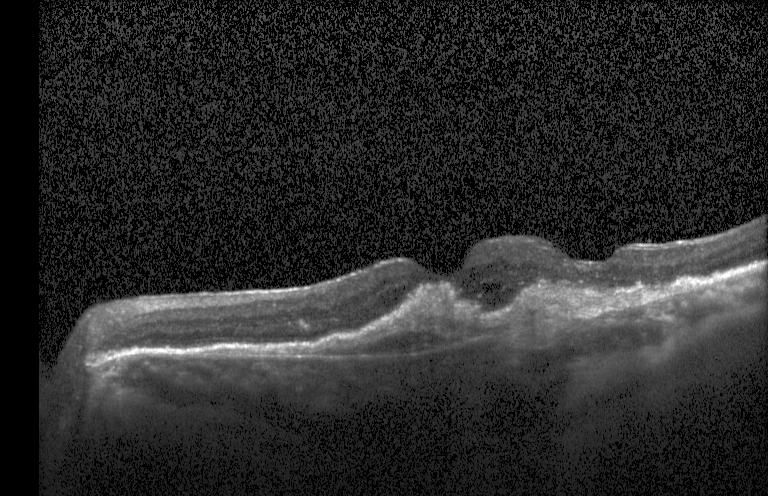

Retinal OCT cross-section, SD-OCT — The scan shows a choroidal neovascular membrane.